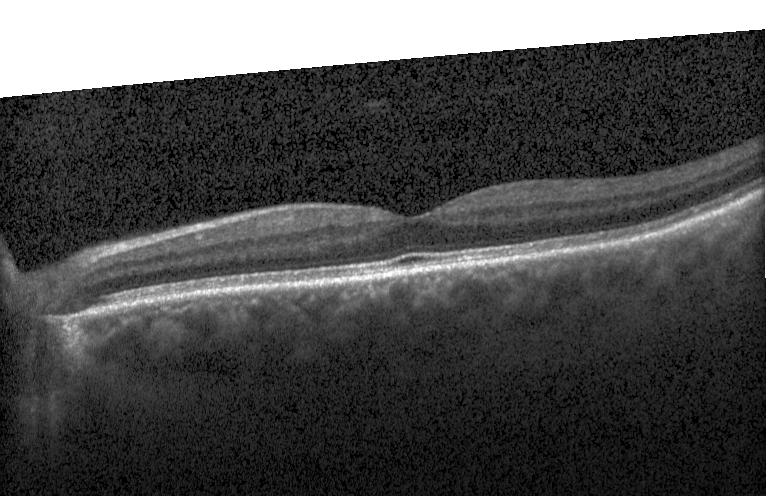

Spectral-domain optical coherence tomography · OCT line scan · through the macula — OCT finding: no CNV, no DME, and no drusen.